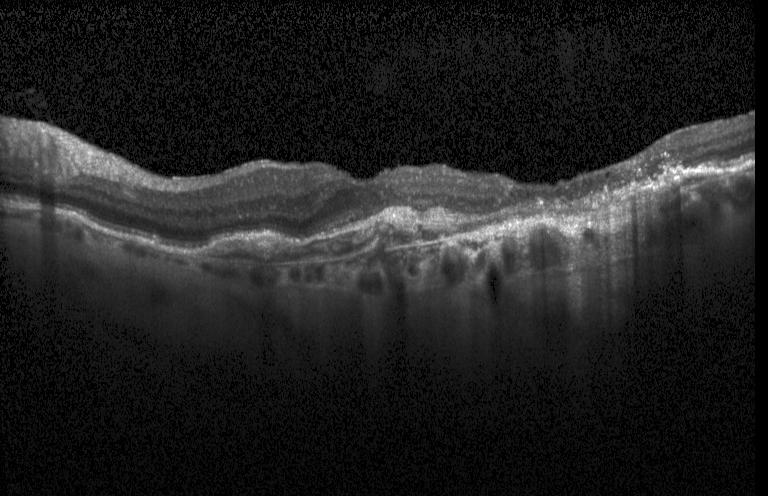

Impression: a choroidal neovascular membrane.